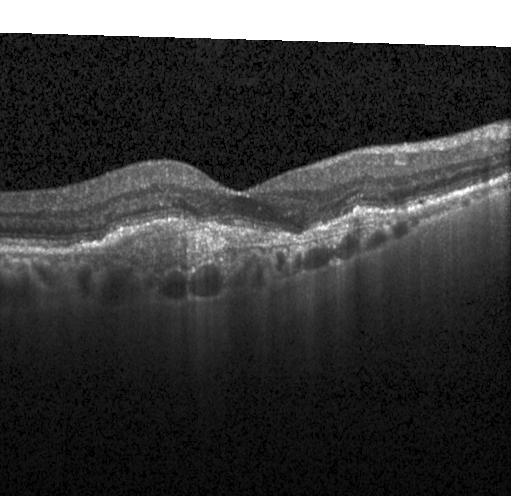
Diagnosis: choroidal neovascularization (CNV).